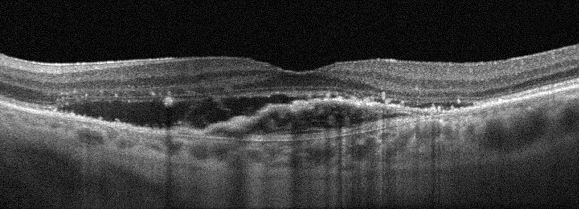
OCT B-scan · oculus sinister — Finding: AMD.